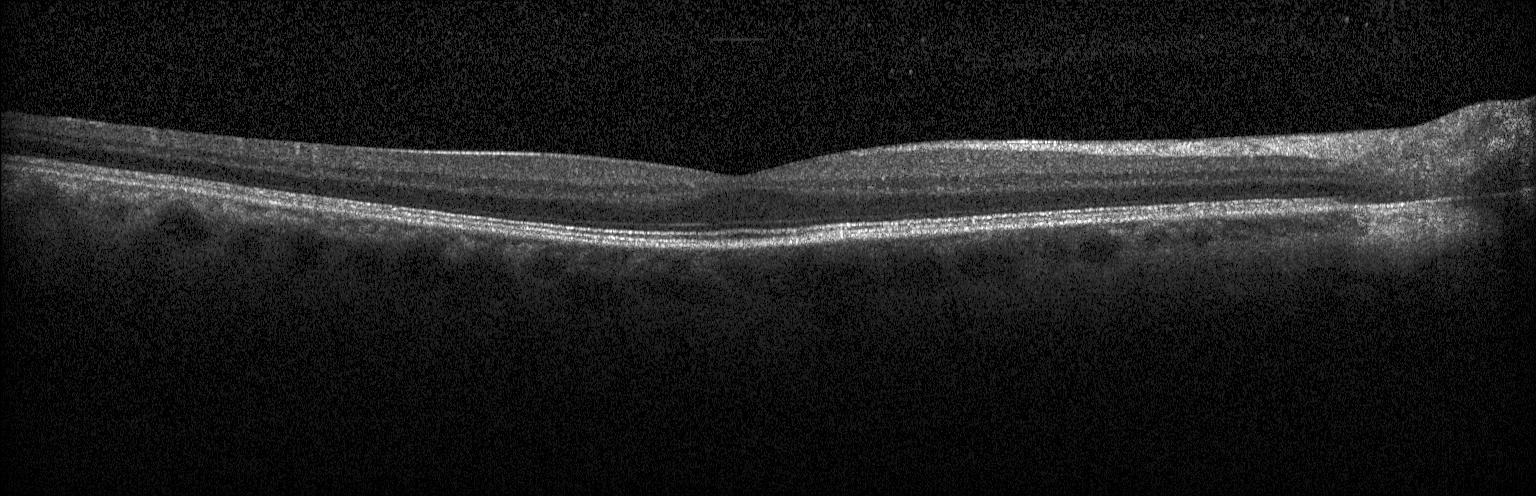
Spectral-domain OCT B-scan: neither choroidal neovascularization, diabetic macular edema, nor drusen.